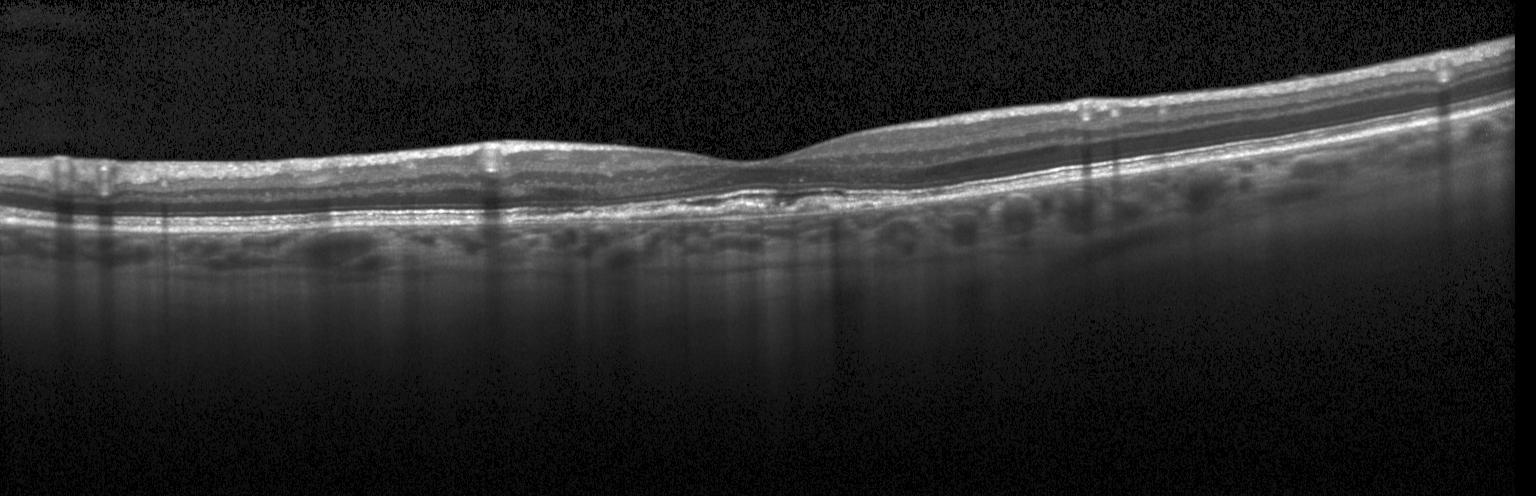 Instrument: Heidelberg Spectralis; SD-OCT; horizontal scan through the fovea; OCT line scan. Finding: a choroidal neovascular membrane.